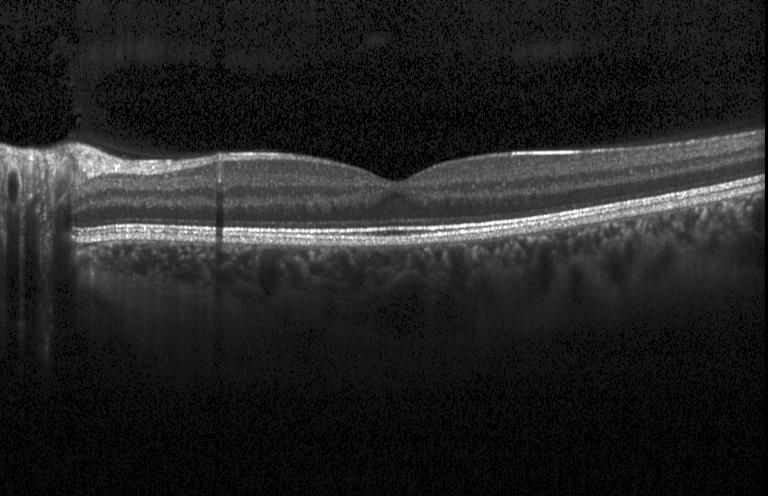 Macular scan. Spectral-domain OCT. OCT B-scan
Dx: no choroidal neovascularization, diabetic macular edema, or drusen.